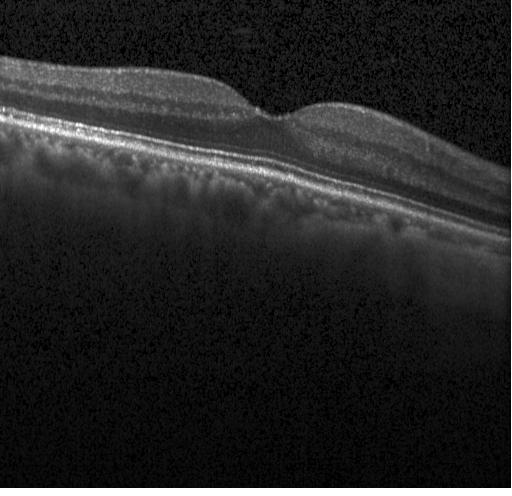
OCT line scan — Assessment: no choroidal neovascularization, diabetic macular edema, or drusen.